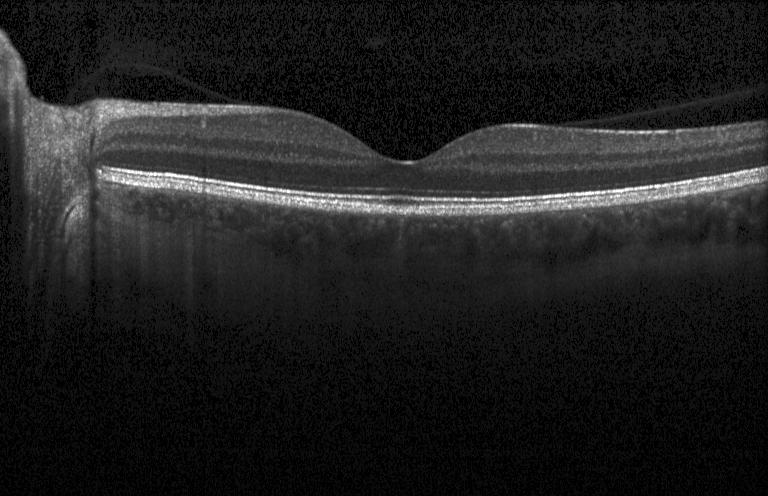

OCT line scan. Diagnosis: no evidence of choroidal neovascularization, diabetic macular edema, or drusen.